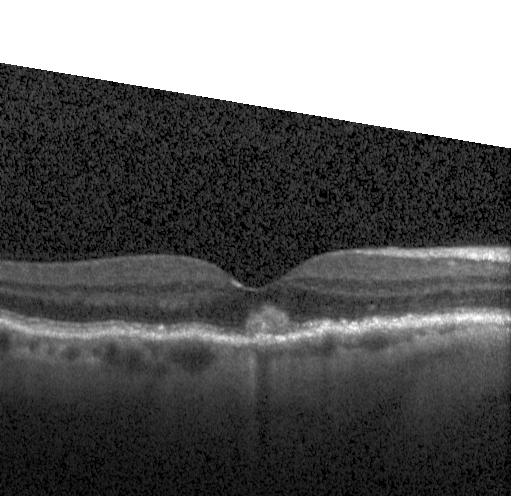

SD-OCT; optical coherence tomography scan
This B-scan demonstrates multiple drusen.